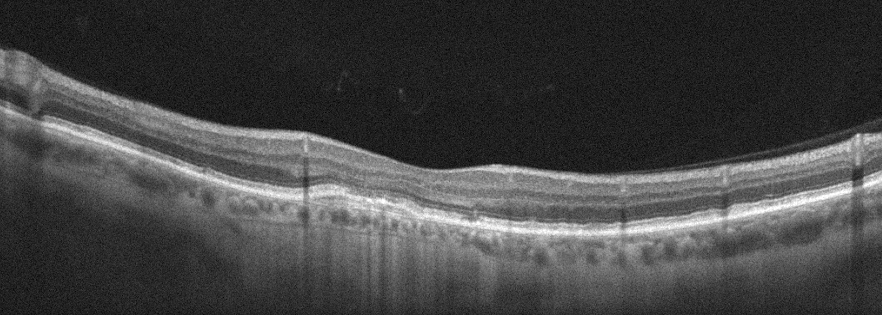

Oculus dexter · retinal OCT B-scan — Diagnosis: age-related macular degeneration.